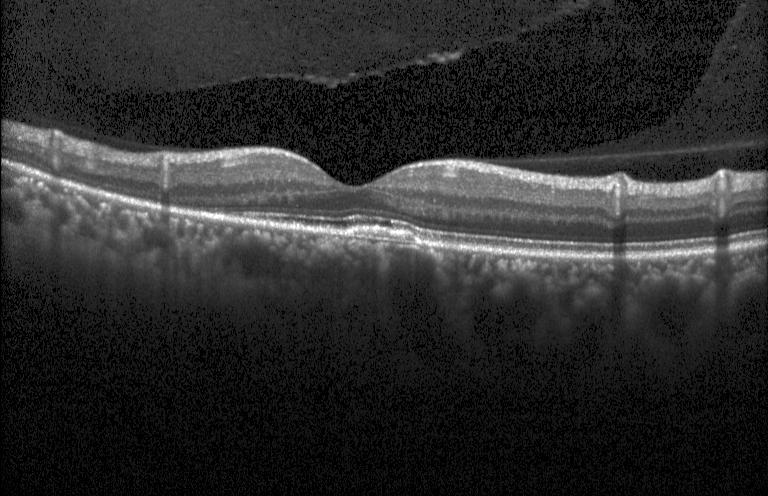 This B-scan demonstrates choroidal neovascularization.